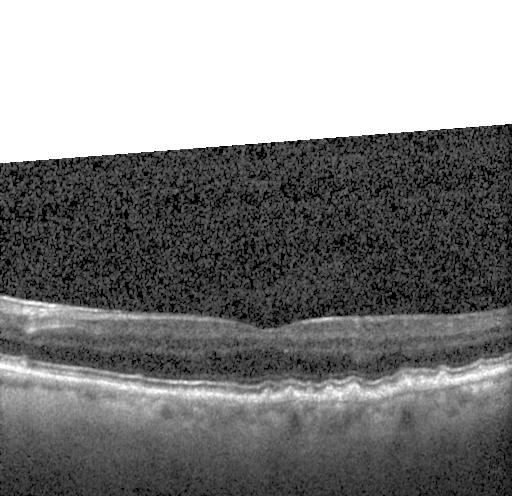
Retinal OCT cross-section, SD-OCT, Heidelberg Spectralis OCT system, centered on the fovea.
Macular OCT: multiple drusen.